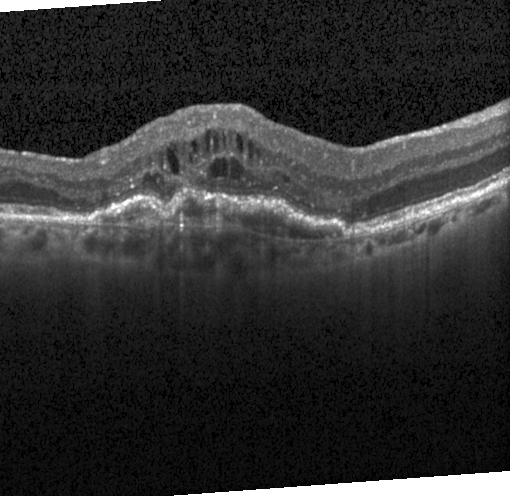

Horizontal scan through the fovea; SD-OCT; instrument: Heidelberg Spectralis; optical coherence tomography B-scan. This B-scan demonstrates choroidal neovascularization.